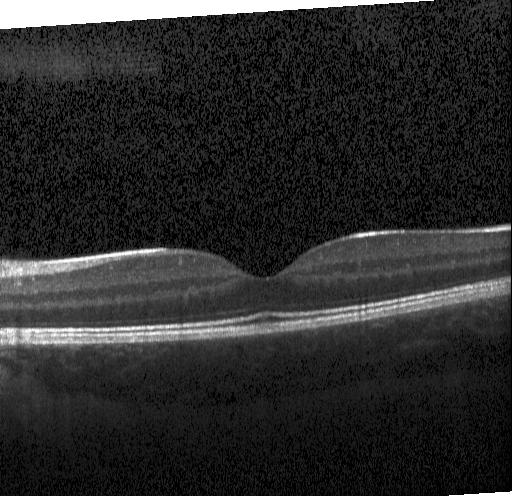
Through the macula; retinal OCT cross-section.
Finding: neither choroidal neovascularization, diabetic macular edema, nor drusen.